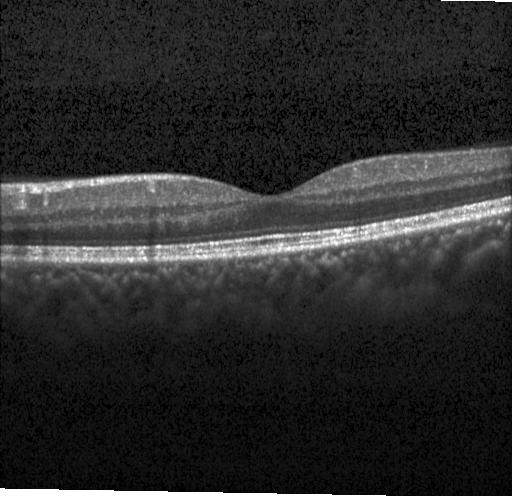 No CNV, DME, or drusen.